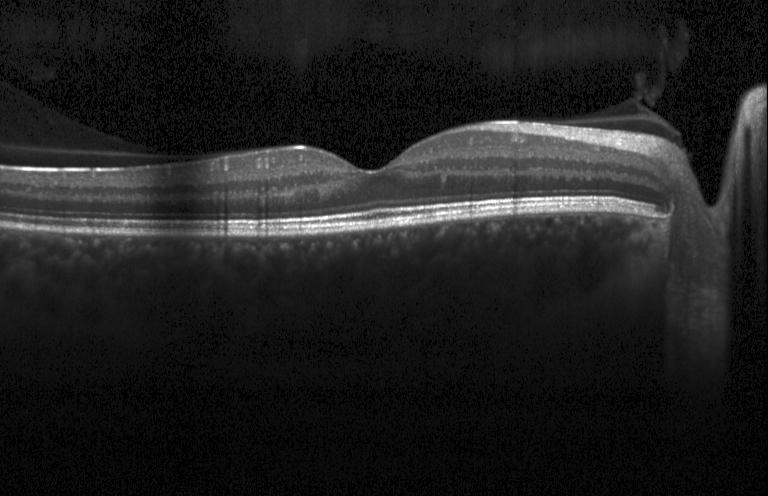
Acquired on a Heidelberg Spectralis, spectral-domain OCT, through the macula, OCT line scan.
OCT finding: no CNV, DME, or drusen.